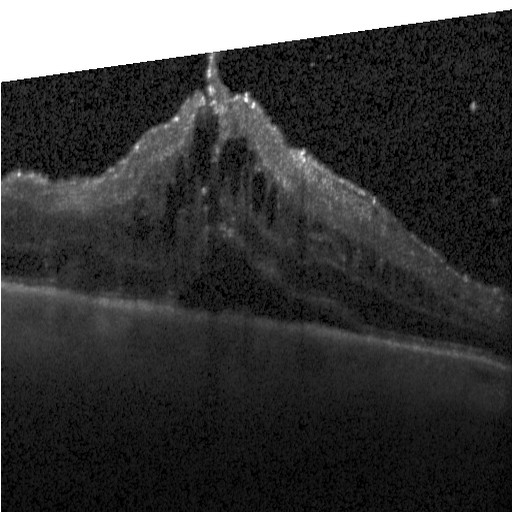
Spectral-domain optical coherence tomography, centered on the fovea, Heidelberg Spectralis OCT system, optical coherence tomography B-scan
Diabetic macular edema (DME).